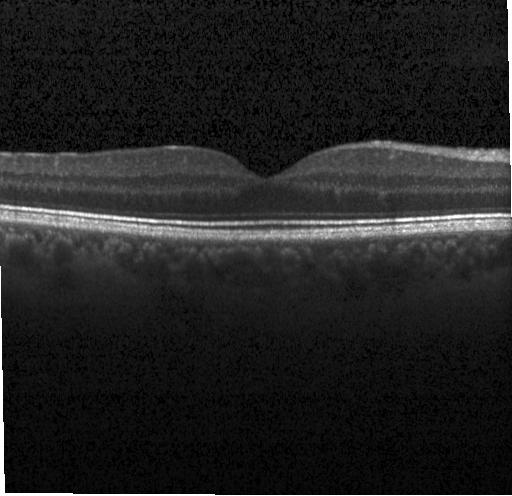 SD-OCT, OCT B-scan — OCT finding: no evidence of CNV, DME, or drusen.